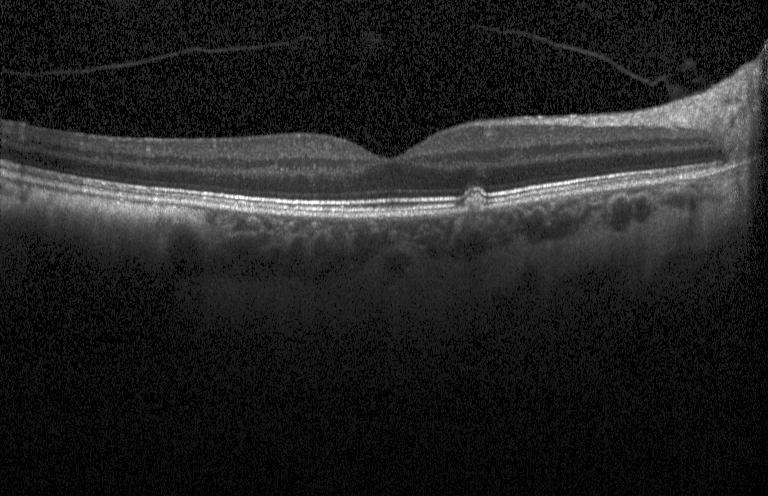 OCT B-scan. Acquired on a Heidelberg Spectralis. Spectral-domain OCT. Impression: sub-RPE drusenoid deposits.